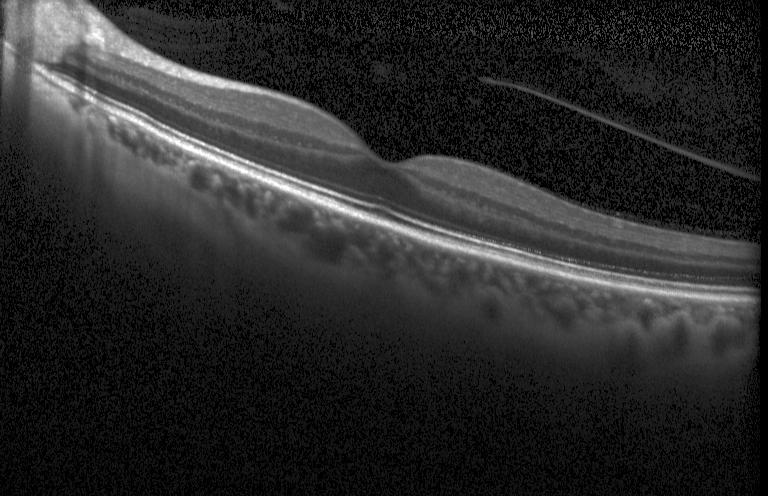 SD-OCT; OCT B-scan; fovea-centered.
Impression: no evidence of CNV, DME, or drusen.